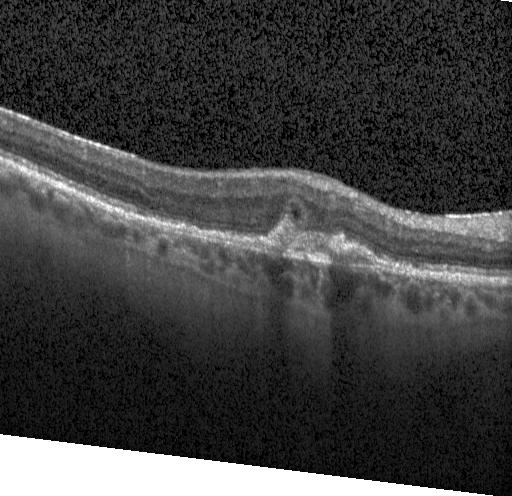

Heidelberg Spectralis, SD-OCT, OCT B-scan.
Diagnosis: a choroidal neovascular membrane.